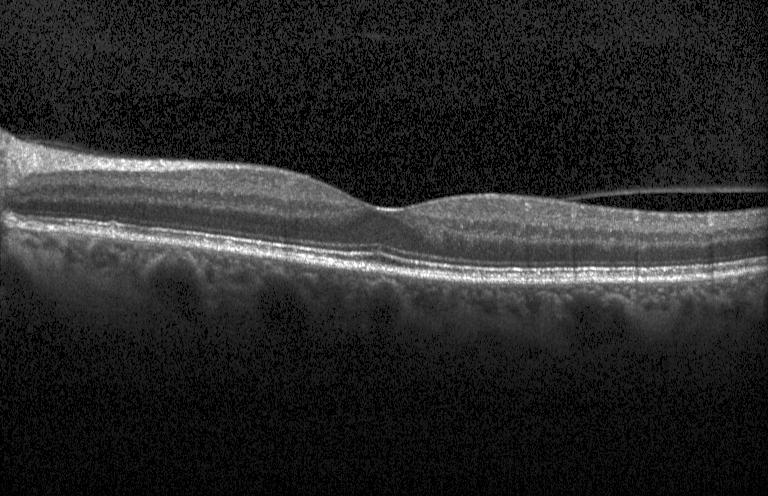
Spectral-domain optical coherence tomography; Heidelberg Spectralis; OCT line scan — Drusen.